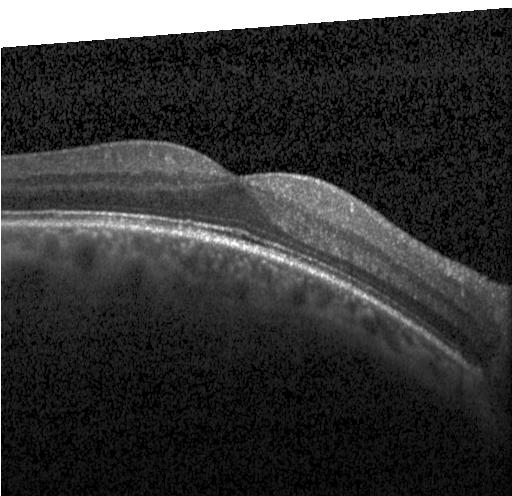

Impression: no CNV, DME, or drusen.